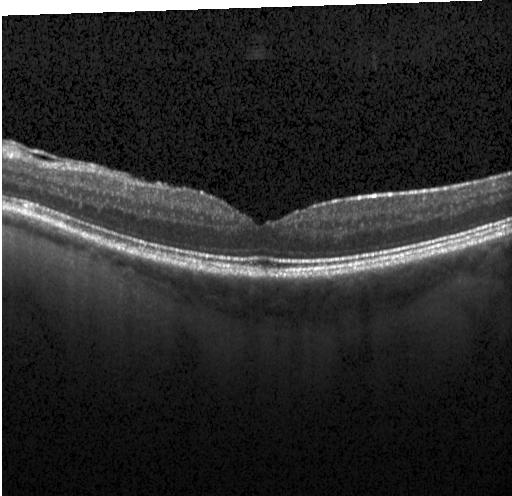 Retinal OCT cross-section · macular scan
OCT finding: no CNV, DME, or drusen.